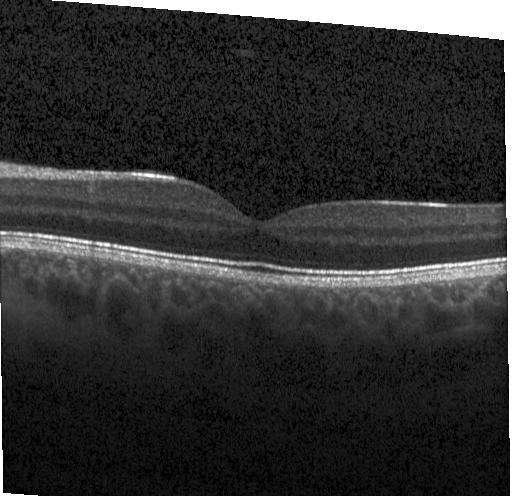 Diagnosis: neither choroidal neovascularization, diabetic macular edema, nor drusen.